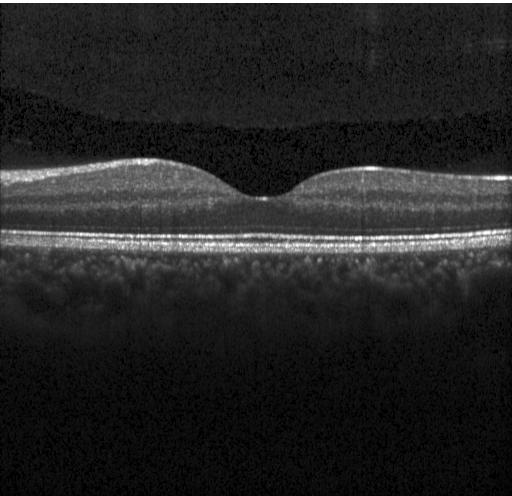 OCT line scan. The scan shows no choroidal neovascularization, diabetic macular edema, or drusen.